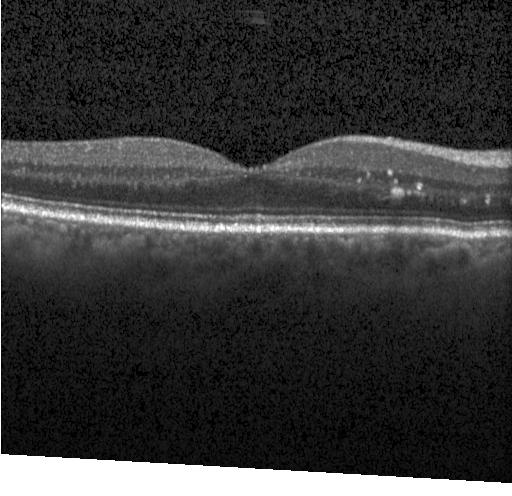
Diagnosis: no choroidal neovascularization, no diabetic macular edema, and no drusen.